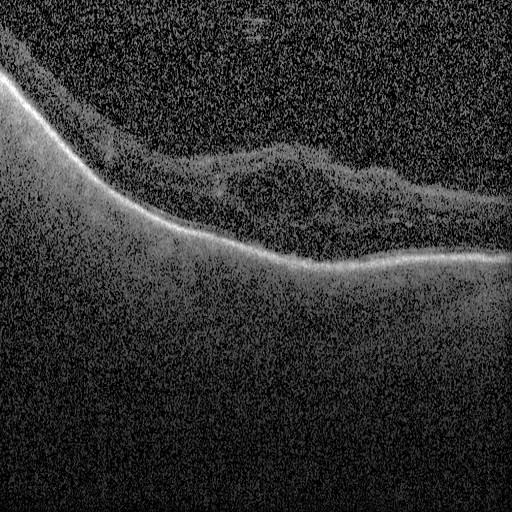

Acquired on a Heidelberg Spectralis; OCT B-scan; fovea-centered; spectral-domain optical coherence tomography — The scan shows diabetic macular edema.